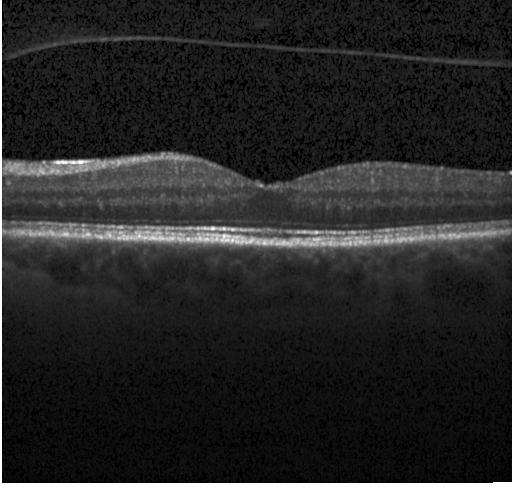 OCT B-scan — Diagnosis: no choroidal neovascularization, diabetic macular edema, or drusen.